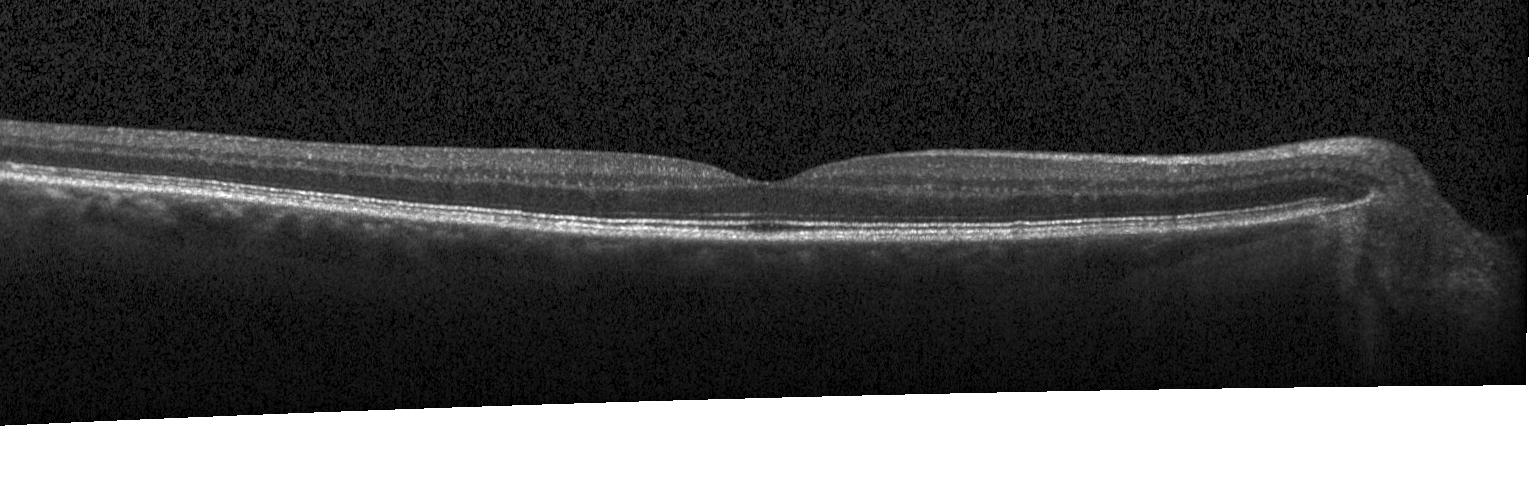

Spectral-domain optical coherence tomography; retinal OCT B-scan; through the macula; Heidelberg Spectralis OCT system
Dx: no evidence of CNV, DME, or drusen.